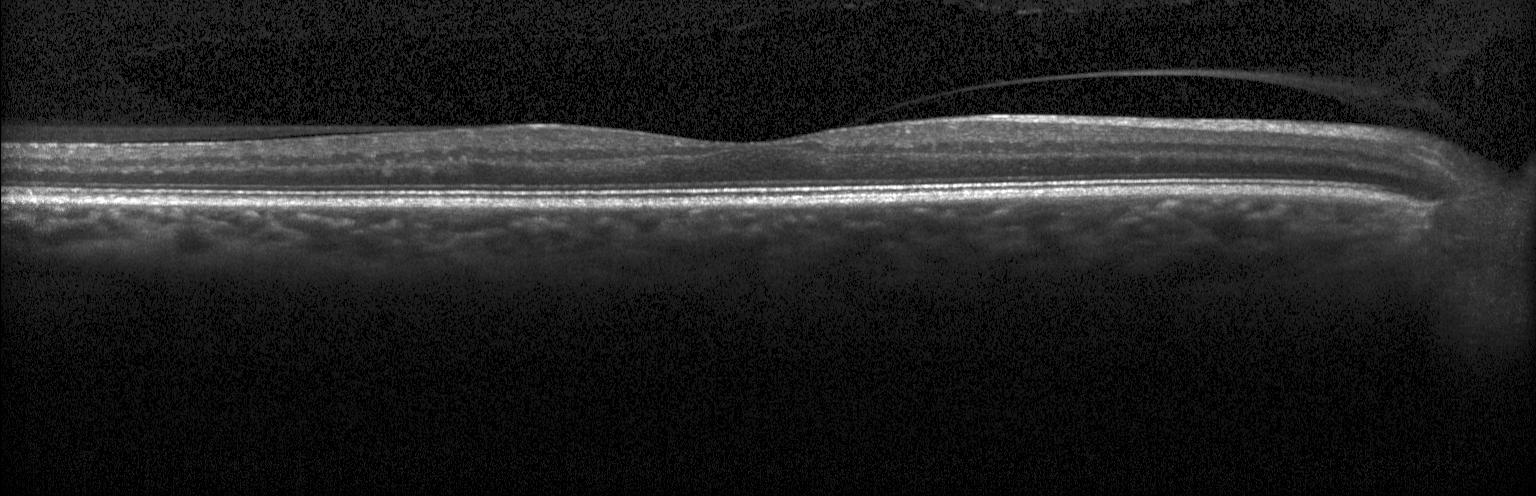

Optical coherence tomography B-scan · instrument: Heidelberg Spectralis · fovea-centered — Macular OCT: no choroidal neovascularization, diabetic macular edema, or drusen.